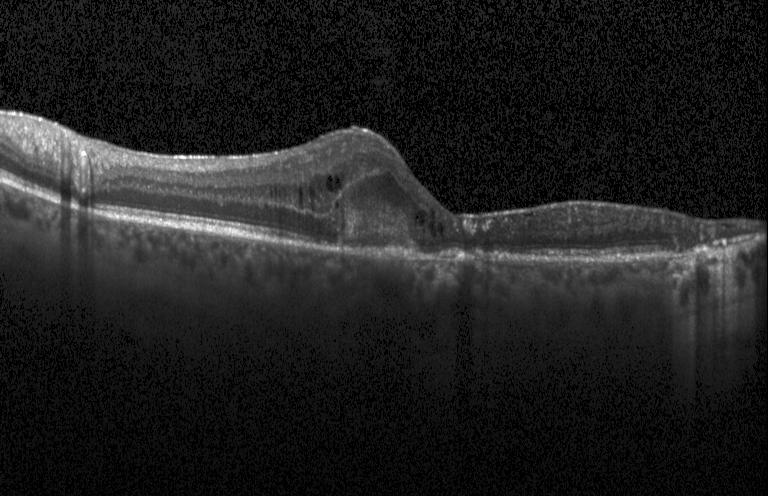

Impression: a choroidal neovascular membrane.